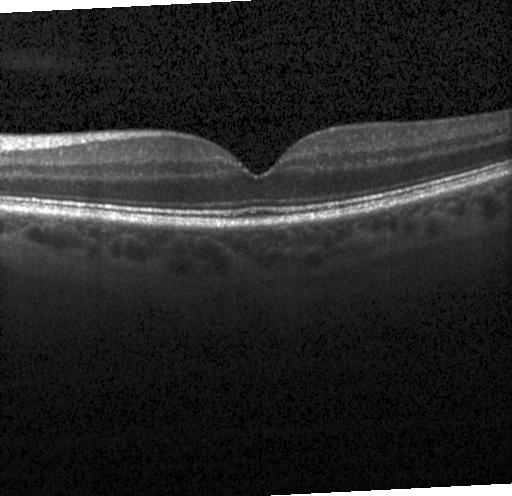 Fovea-centered, Heidelberg Spectralis OCT system, OCT B-scan
This B-scan demonstrates neither choroidal neovascularization, diabetic macular edema, nor drusen.